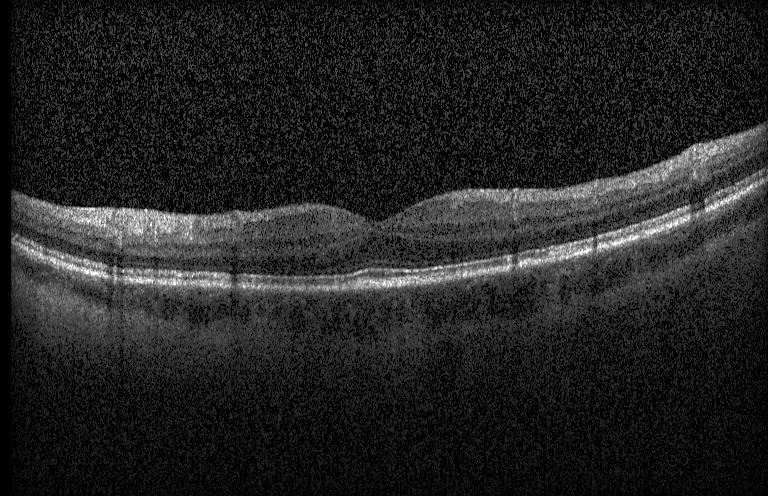 Instrument: Heidelberg Spectralis · OCT B-scan — Impression: no evidence of choroidal neovascularization, diabetic macular edema, or drusen.